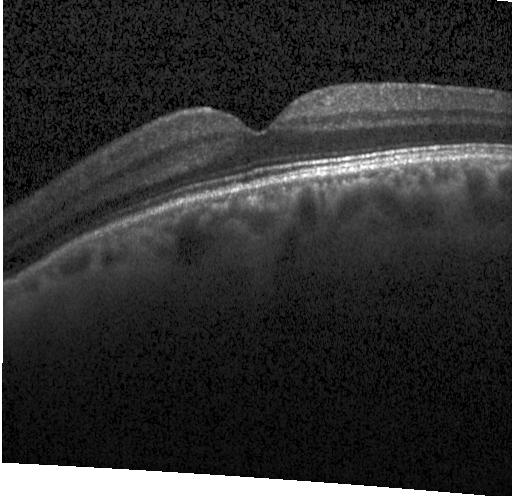

SD-OCT. Centered on the fovea. Acquired on a Heidelberg Spectralis. Retinal OCT cross-section — Impression: no choroidal neovascularization, no diabetic macular edema, and no drusen.